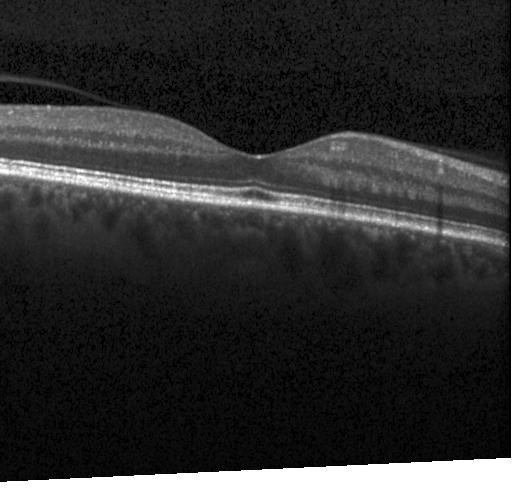

Spectral-domain OCT, OCT B-scan
Impression: neither choroidal neovascularization, diabetic macular edema, nor drusen.